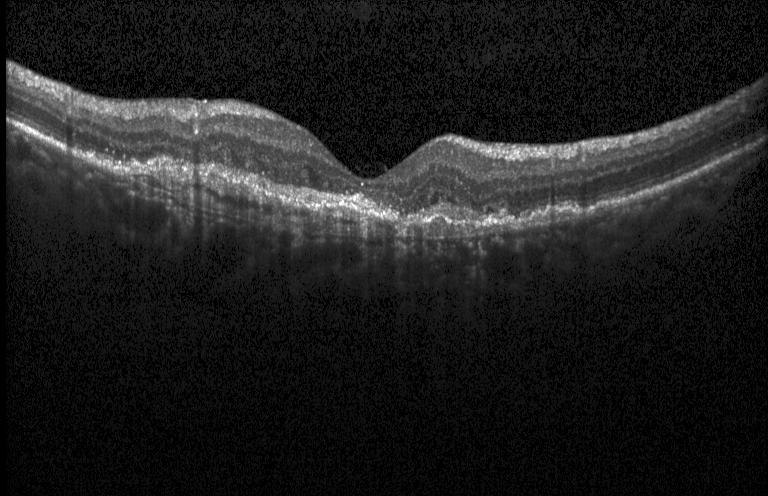 Optical coherence tomography B-scan · spectral-domain OCT · instrument: Heidelberg Spectralis
Dx: choroidal neovascularization.